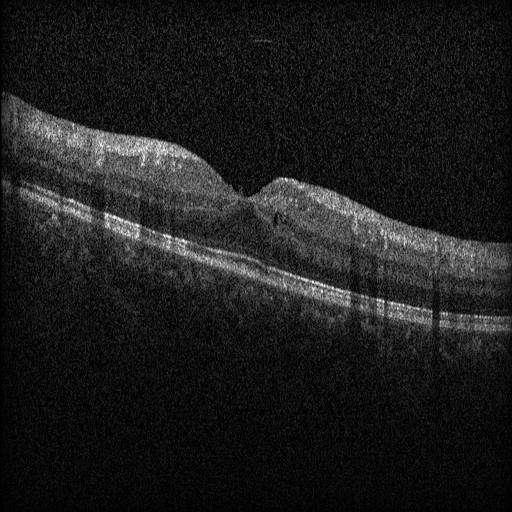 Diagnosis: diabetic macular edema (DME).